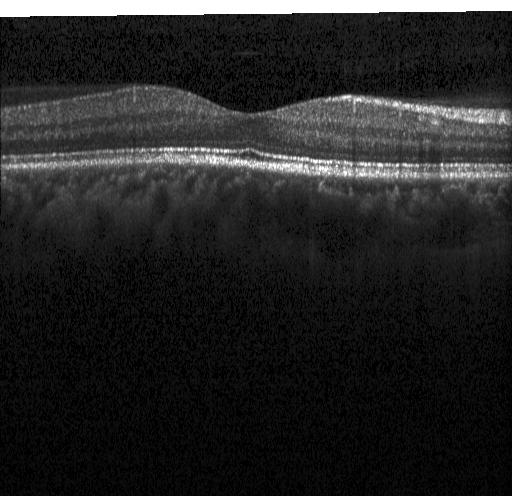

Heidelberg Spectralis, retinal OCT cross-section, spectral-domain OCT, fovea-centered — Dx: no evidence of choroidal neovascularization, diabetic macular edema, or drusen.